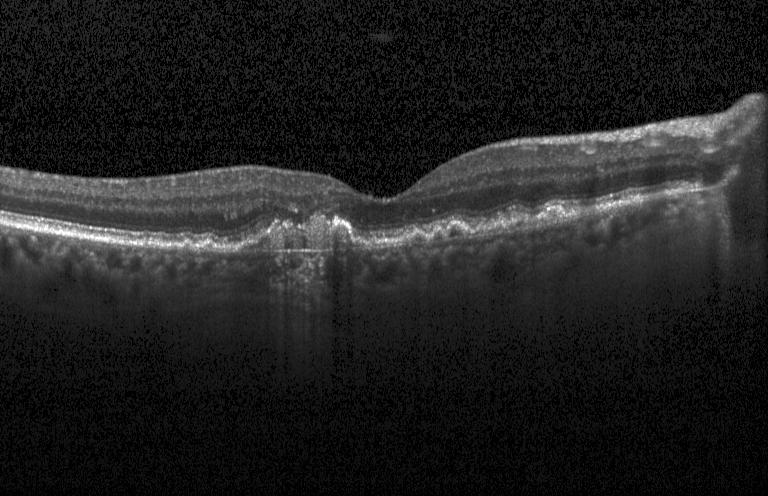
Fovea-centered. Retinal OCT cross-section. Acquired on a Heidelberg Spectralis
Dx: a choroidal neovascular membrane.